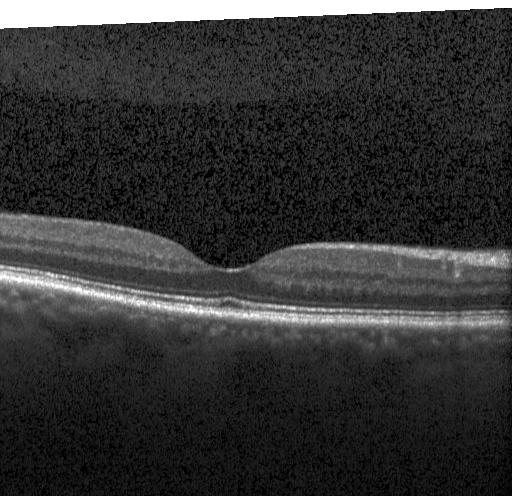 Retinal OCT B-scan · Heidelberg Spectralis OCT system · spectral-domain optical coherence tomography.
The scan shows no evidence of choroidal neovascularization, diabetic macular edema, or drusen.